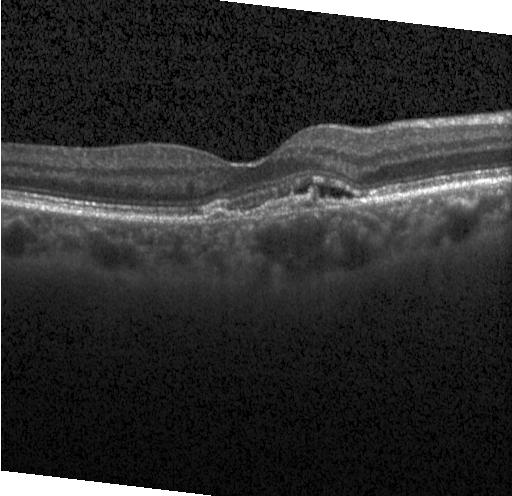 Macular OCT: a choroidal neovascular membrane.